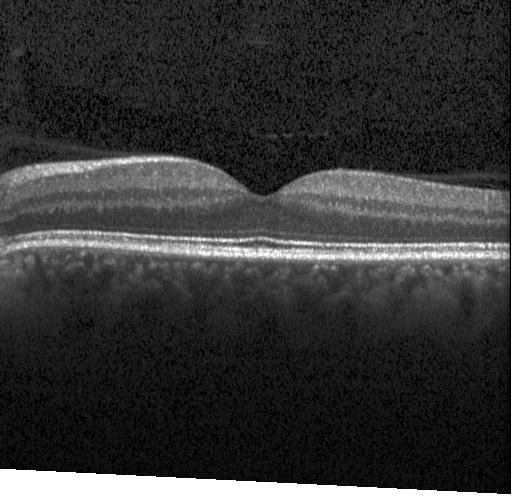 Heidelberg Spectralis OCT system. Centered on the fovea. Optical coherence tomography B-scan. SD-OCT.
Assessment: neither choroidal neovascularization, diabetic macular edema, nor drusen.